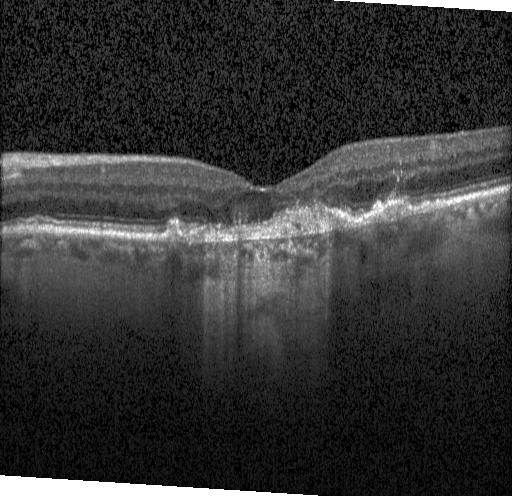

Spectral-domain OCT B-scan: CNV.